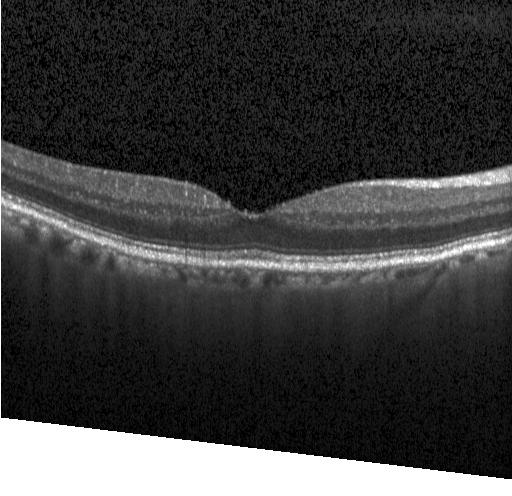
Retinal OCT cross-section
No choroidal neovascularization, no diabetic macular edema, and no drusen.